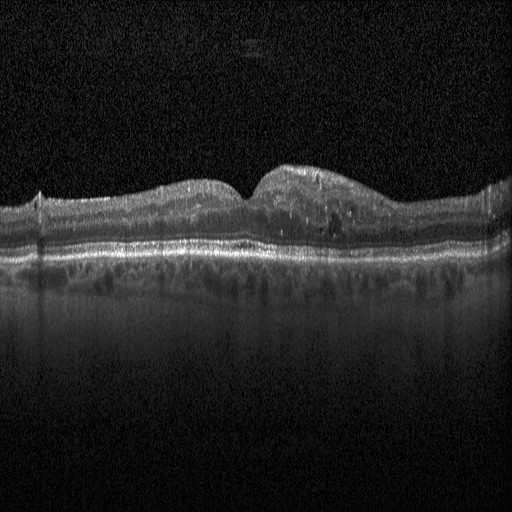

Impression: diabetic macular edema.